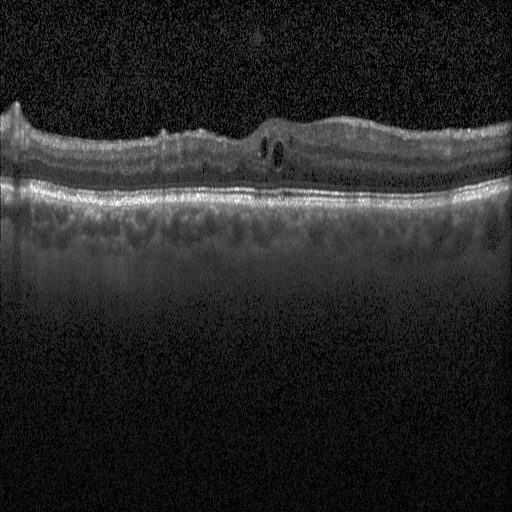
SD-OCT; OCT line scan; fovea-centered
Dx: DME.